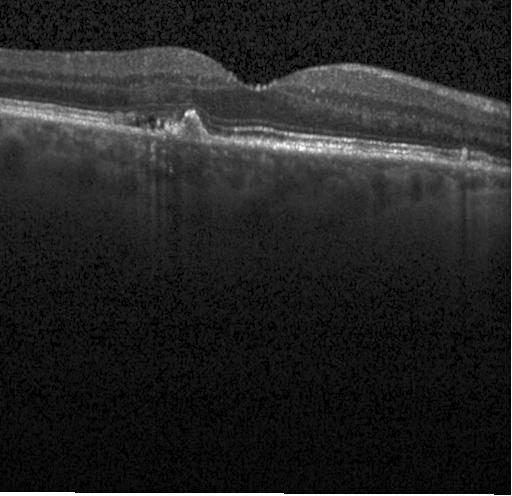
Fovea-centered · Heidelberg Spectralis OCT system · OCT line scan · spectral-domain optical coherence tomography — A choroidal neovascular membrane.